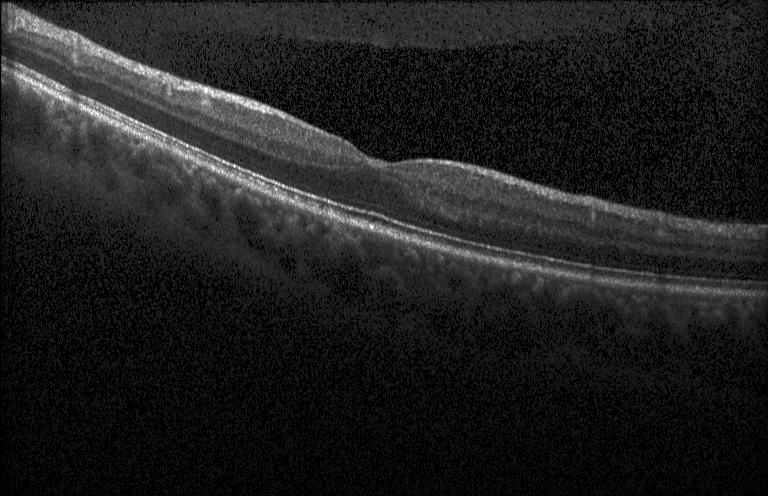

Finding: neither CNV, DME, nor drusen.